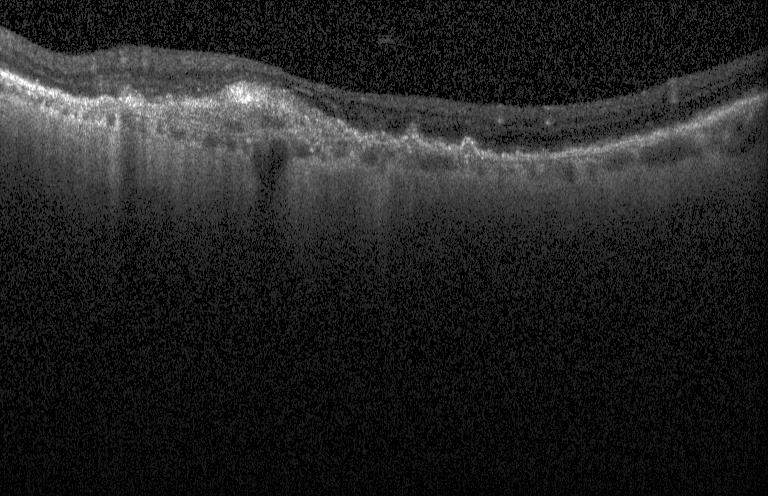

Optical coherence tomography B-scan, acquired on a Heidelberg Spectralis, through the macula, spectral-domain OCT — This B-scan demonstrates choroidal neovascularization (CNV).